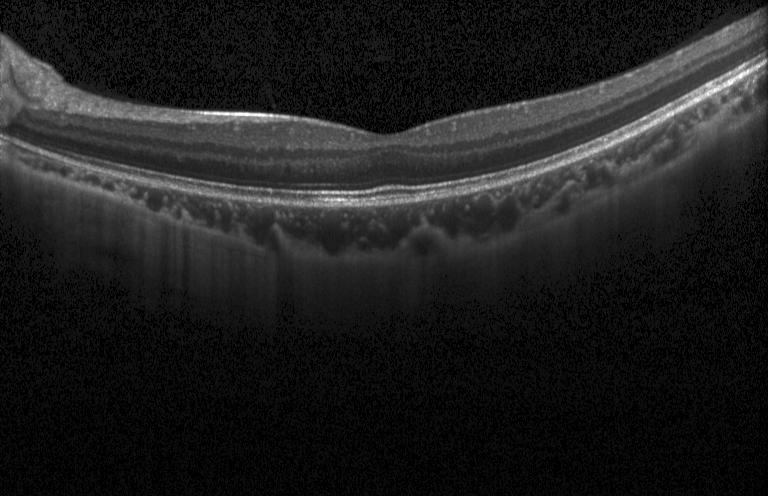
Impression: no evidence of choroidal neovascularization, diabetic macular edema, or drusen.